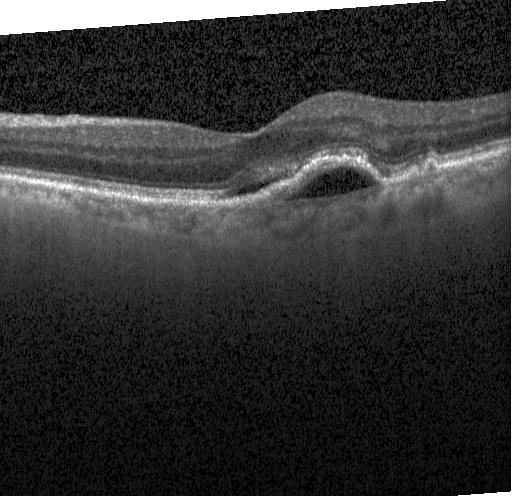

Spectral-domain optical coherence tomography. Retinal OCT B-scan — Finding: choroidal neovascularization.